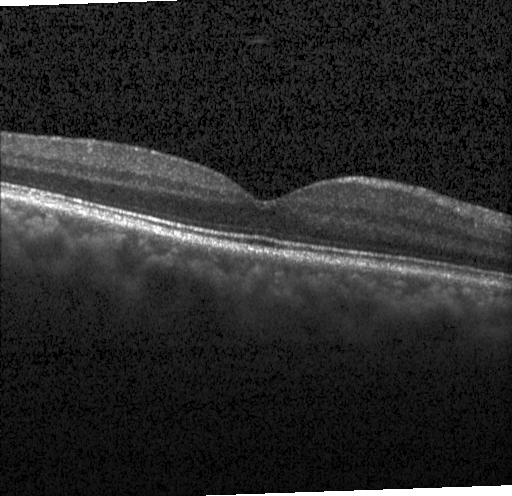

OCT B-scan showing no evidence of choroidal neovascularization, diabetic macular edema, or drusen.